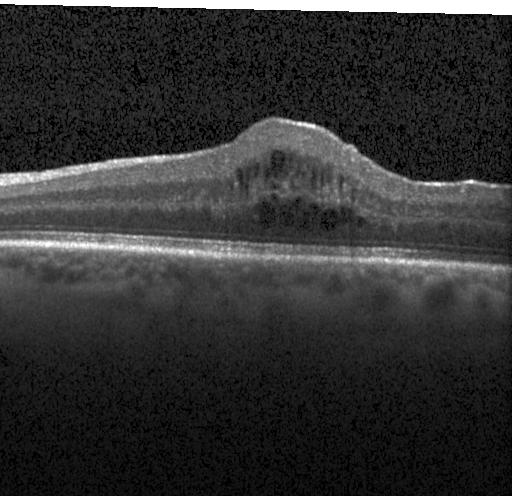 Retinal OCT cross-section.
Dx: diabetic macular edema (DME).